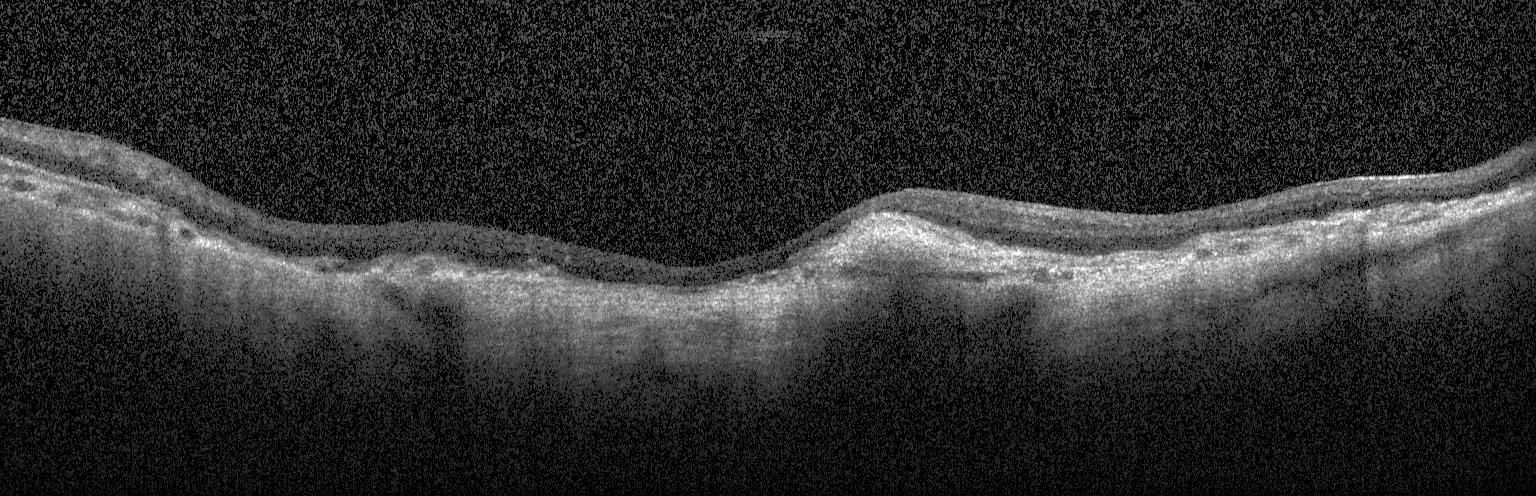
Impression: a choroidal neovascular membrane.